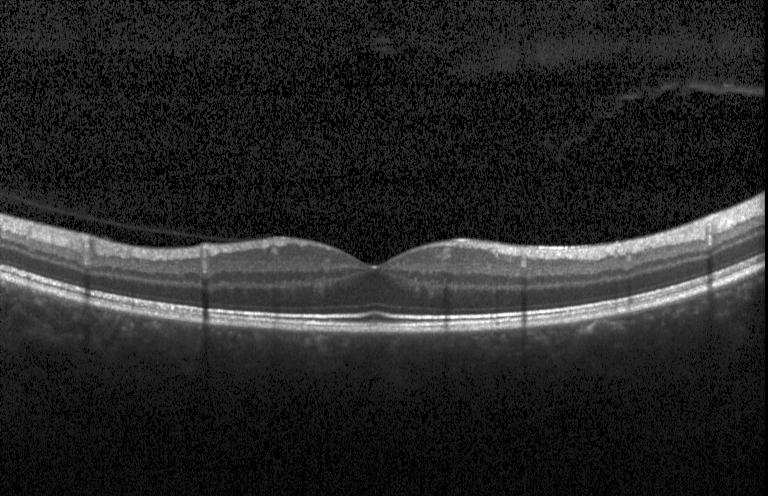 Retinal OCT cross-section showing no evidence of CNV, DME, or drusen.